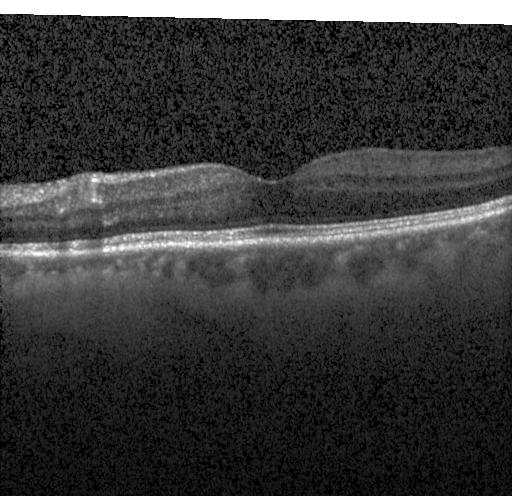

Retinal OCT cross-section. Finding: no CNV, no DME, and no drusen.